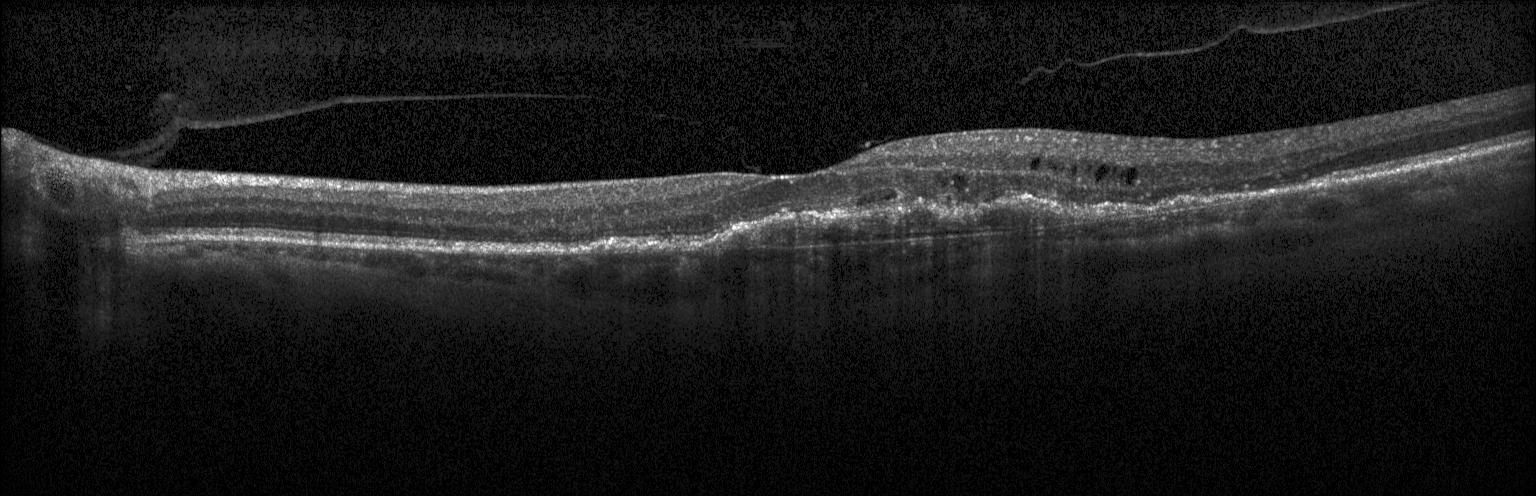

Instrument: Heidelberg Spectralis, macular scan, retinal OCT B-scan
Impression: a choroidal neovascular membrane.